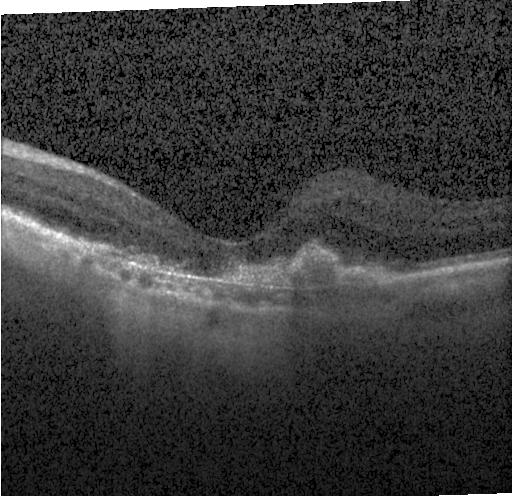
Optical coherence tomography scan · spectral-domain OCT · Heidelberg Spectralis · macular scan.
Finding: choroidal neovascularization.